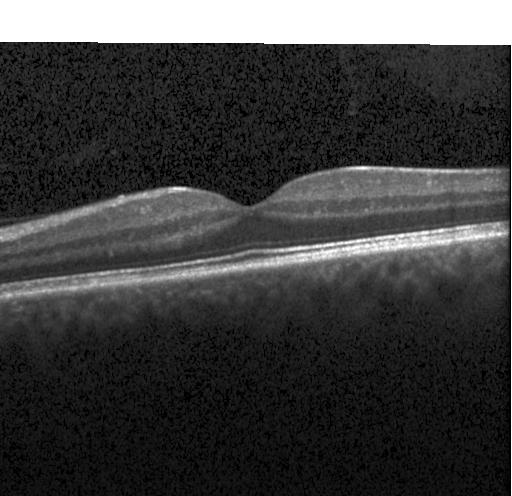

Diagnosis: no CNV, no DME, and no drusen.